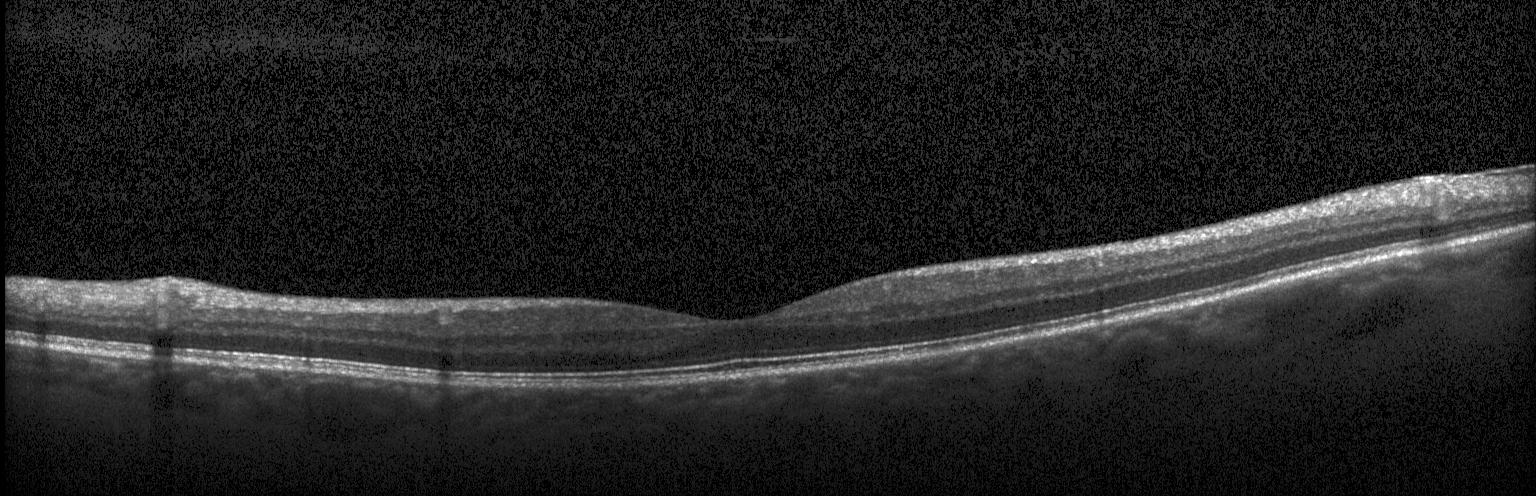

Finding: no evidence of choroidal neovascularization, diabetic macular edema, or drusen.